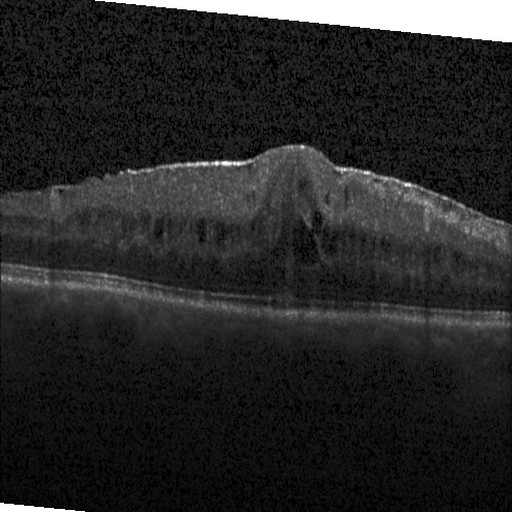 Diagnosis: DME.